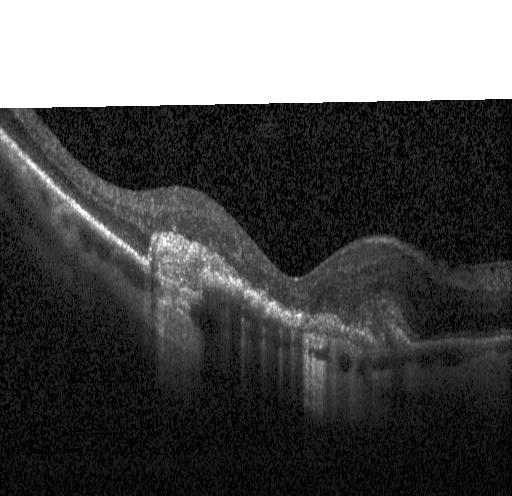
Heidelberg Spectralis, optical coherence tomography B-scan — Finding: choroidal neovascularization (CNV).